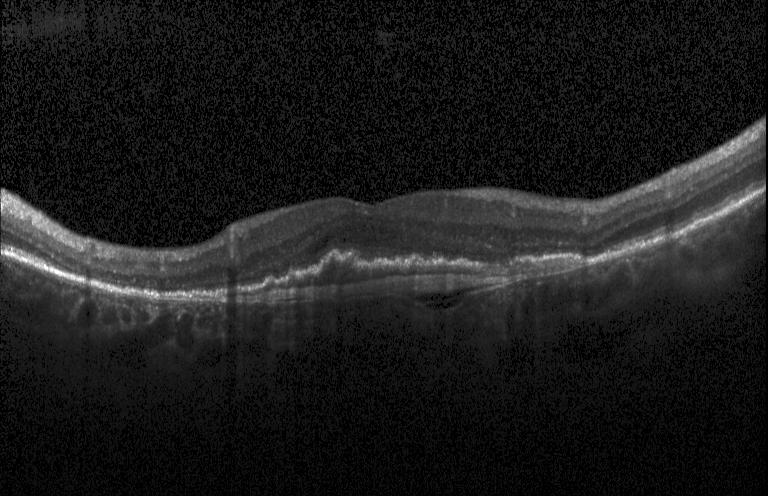 Assessment: choroidal neovascularization (CNV).